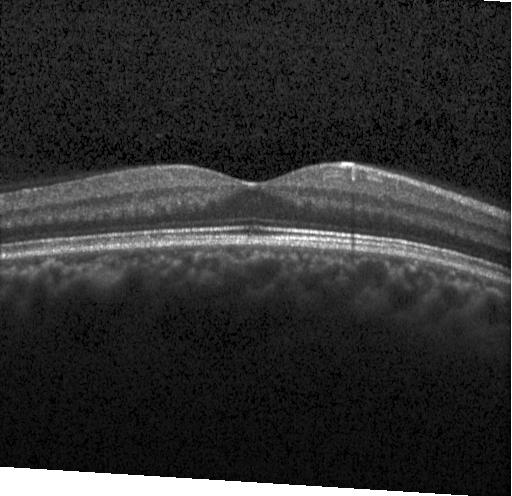 Diagnosis: neither choroidal neovascularization, diabetic macular edema, nor drusen.